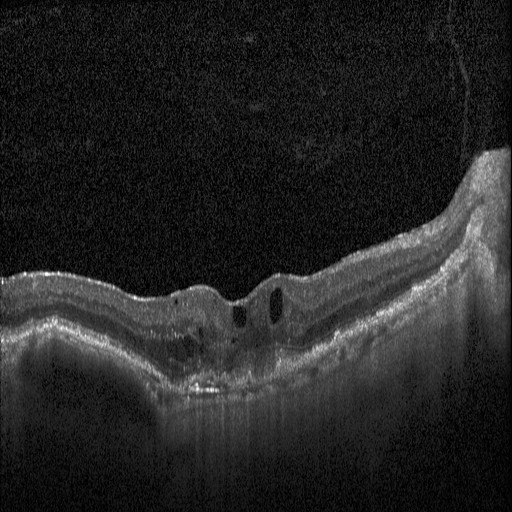
Macular OCT demonstrating DME.